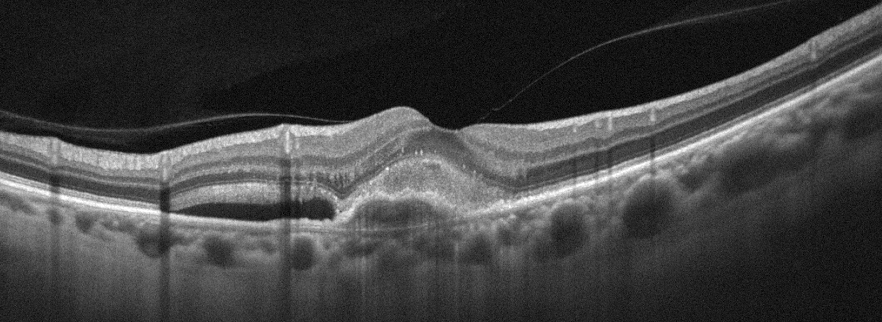
OD; retinal OCT cross-section — The scan shows AMD.